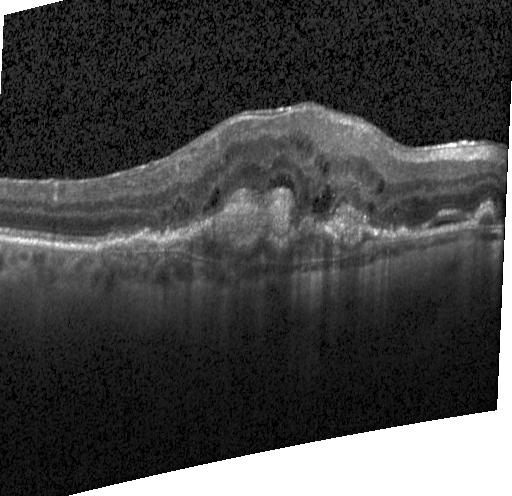

Retinal OCT cross-section showing a choroidal neovascular membrane.